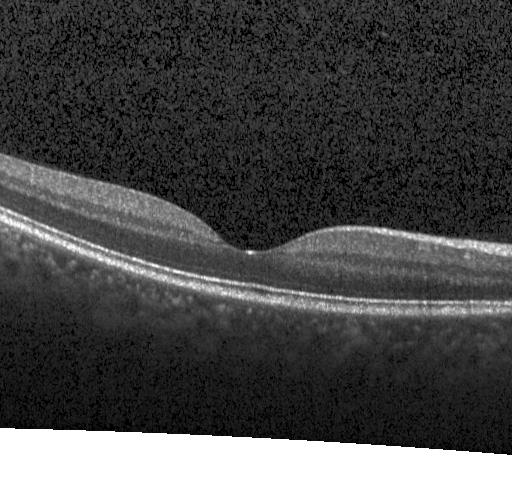
Diagnosis: no evidence of CNV, DME, or drusen.